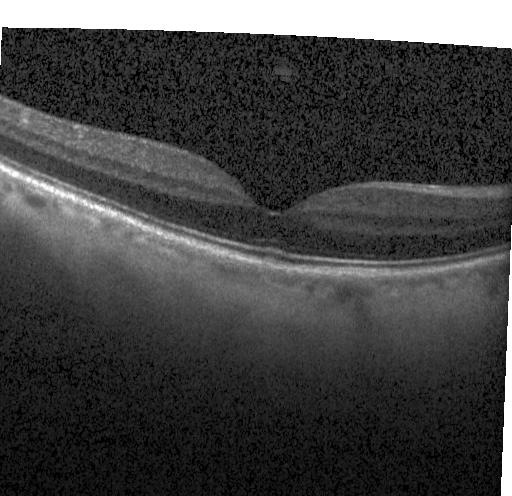

Macular OCT: no evidence of CNV, DME, or drusen.